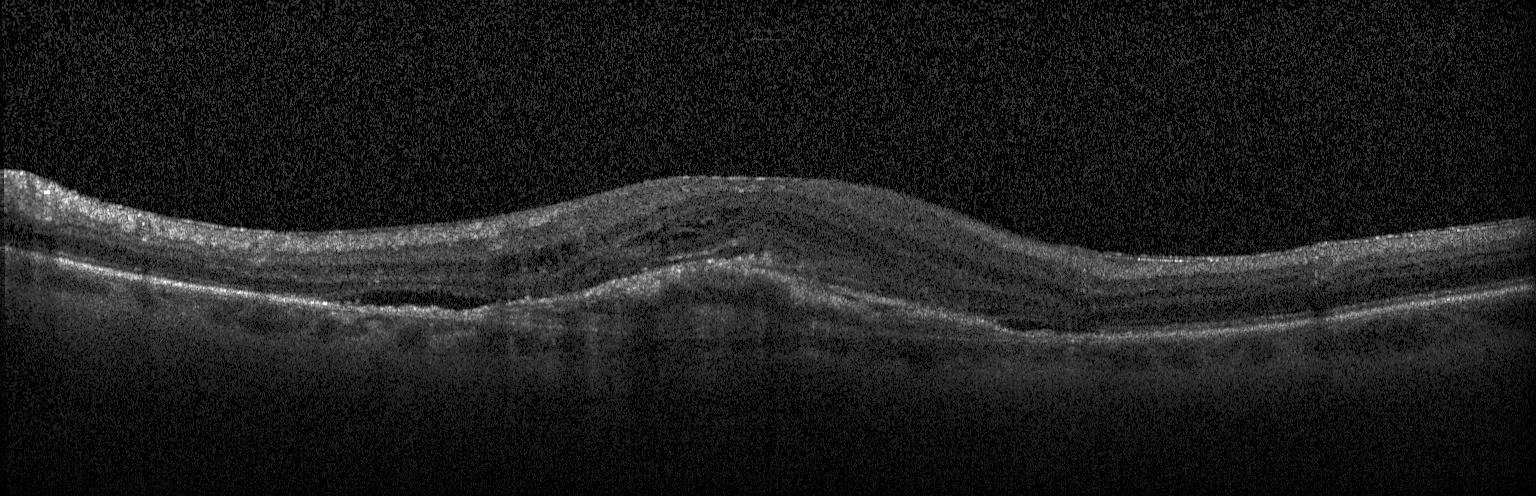
Instrument: Heidelberg Spectralis. Spectral-domain optical coherence tomography. Fovea-centered. Optical coherence tomography B-scan — Diagnosis: a choroidal neovascular membrane.